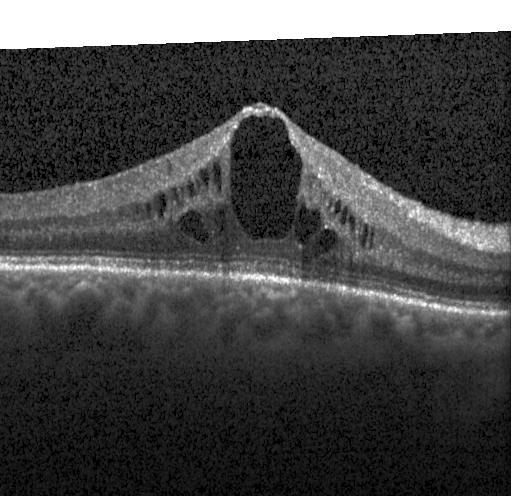 OCT B-scan showing DME.